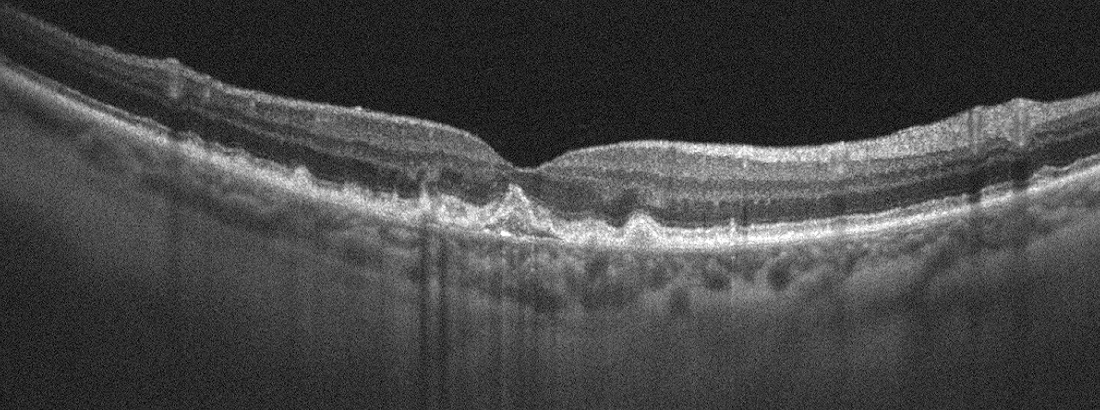
OCT line scan · instrument: Optovue Avanti RTVue XR
Macular OCT: age-related macular degeneration (AMD).